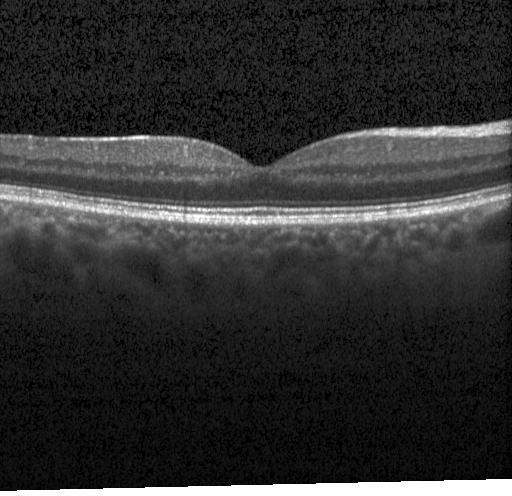 Optical coherence tomography scan.
Dx: no choroidal neovascularization, diabetic macular edema, or drusen.